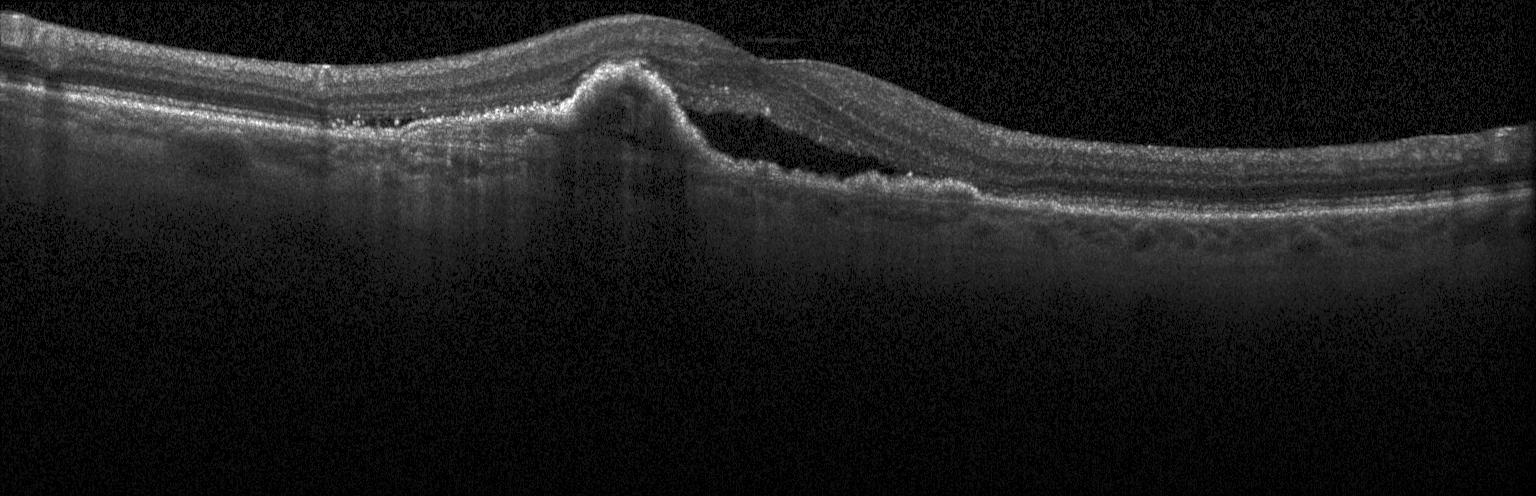

Dx: a choroidal neovascular membrane.